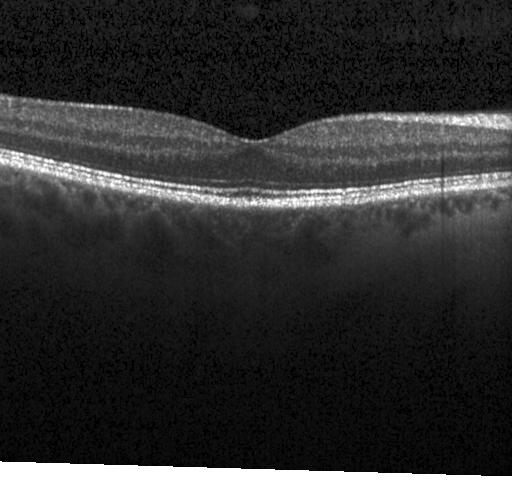

Optical coherence tomography B-scan. Heidelberg Spectralis.
Diagnosis: no evidence of choroidal neovascularization, diabetic macular edema, or drusen.